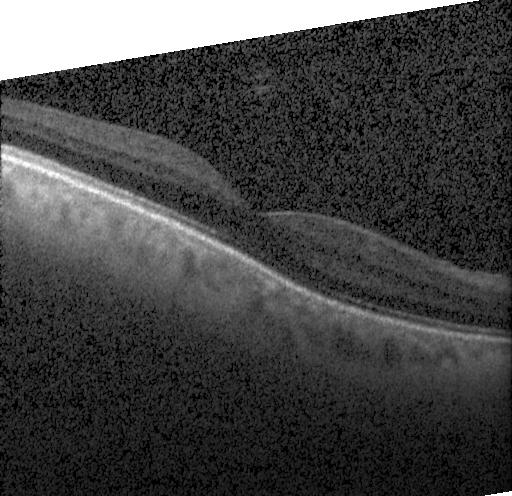
Optical coherence tomography B-scan. Spectral-domain OCT. Macular scan. Instrument: Heidelberg Spectralis
OCT finding: no evidence of choroidal neovascularization, diabetic macular edema, or drusen.